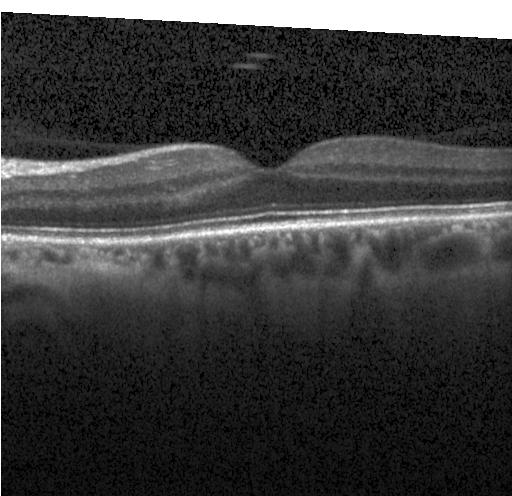

Retinal OCT B-scan. Heidelberg Spectralis
Finding: no evidence of choroidal neovascularization, diabetic macular edema, or drusen.